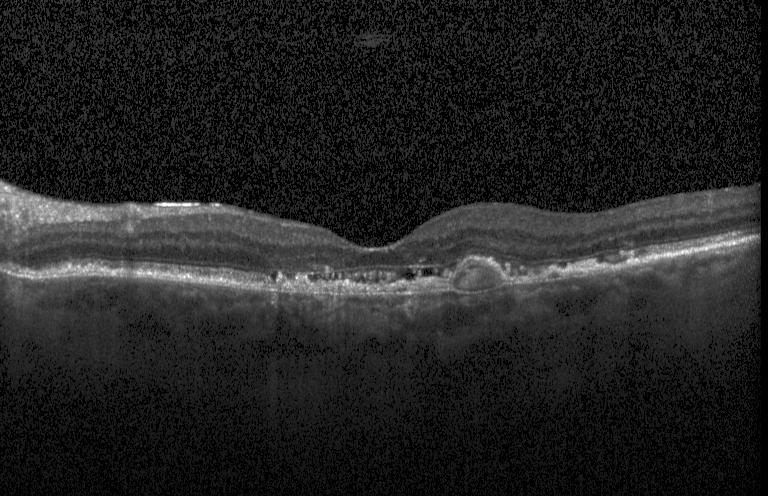

Optical coherence tomography B-scan; fovea-centered
The scan shows a choroidal neovascular membrane.